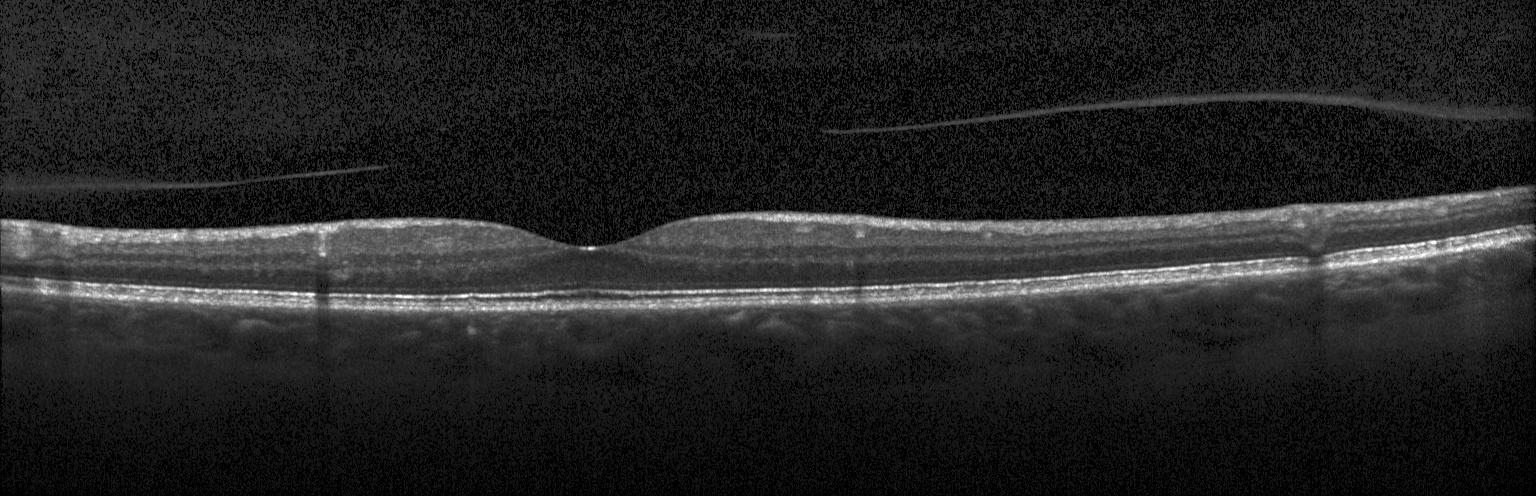 Heidelberg Spectralis, retinal OCT cross-section.
Assessment: no choroidal neovascularization, diabetic macular edema, or drusen.